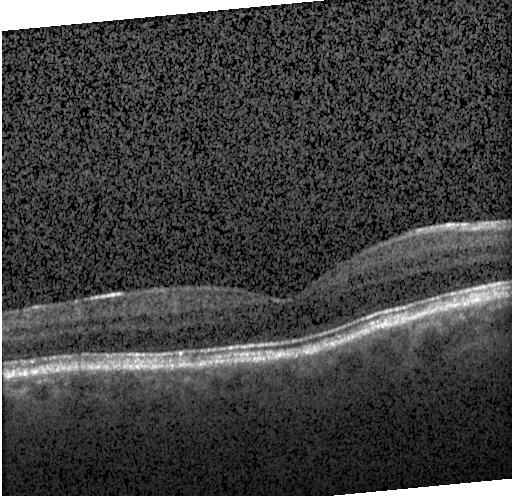
This B-scan demonstrates no choroidal neovascularization, diabetic macular edema, or drusen.